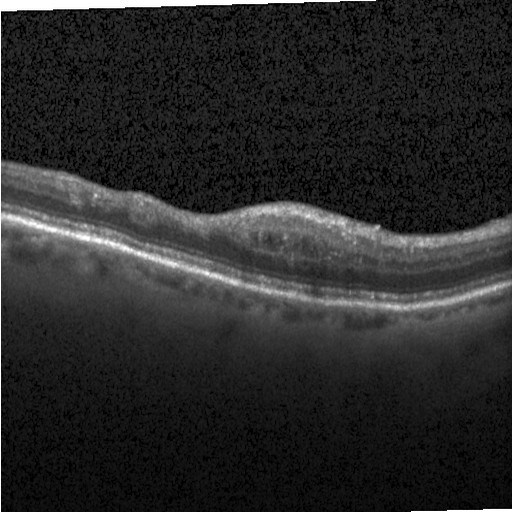

Retinal OCT cross-section; spectral-domain optical coherence tomography — Finding: DME.